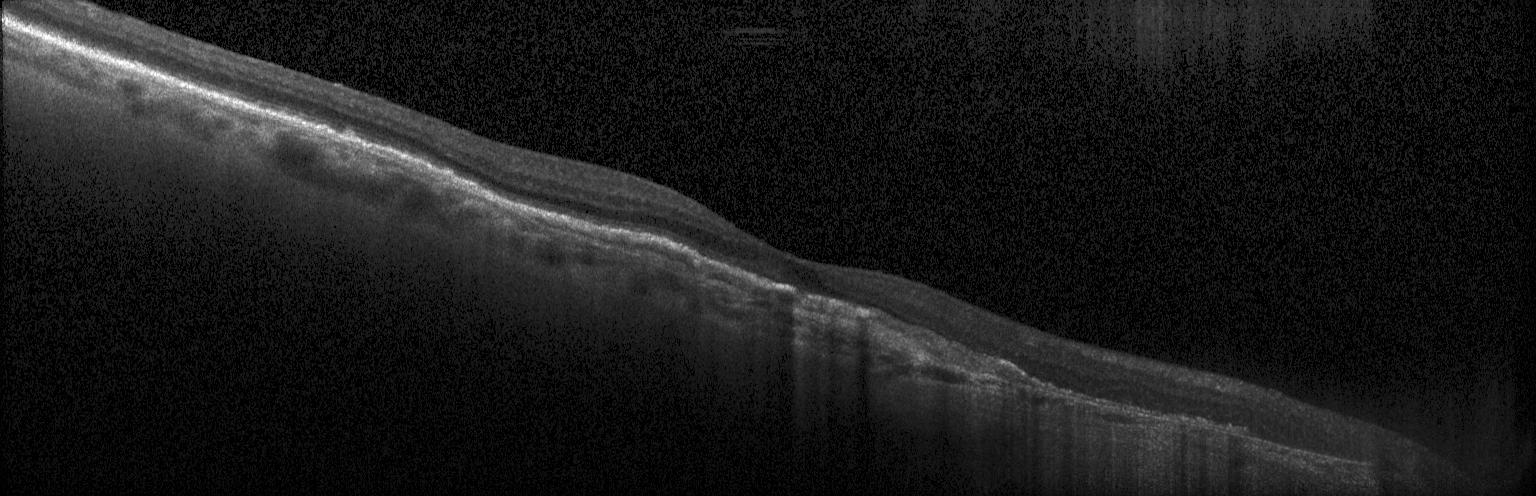
Assessment: a choroidal neovascular membrane.